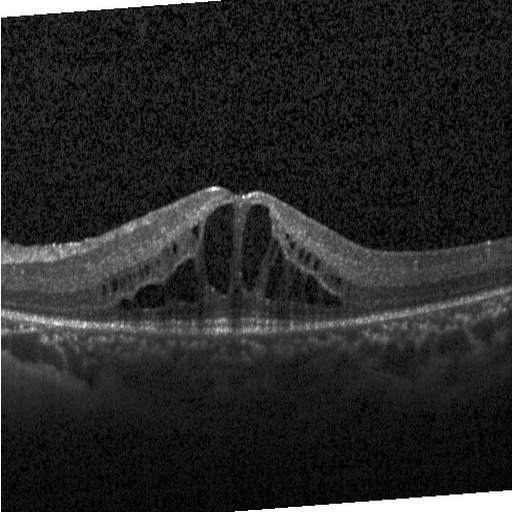

Macular OCT: DME.